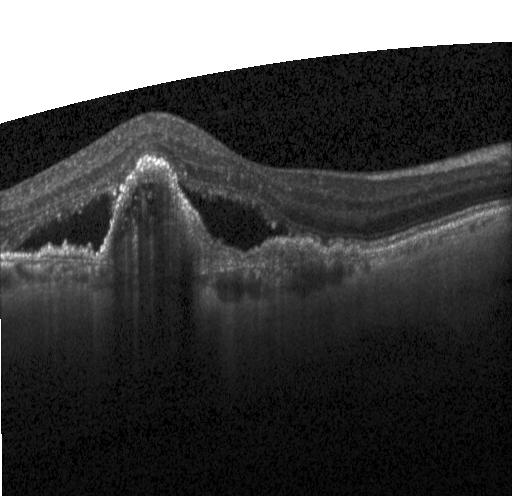

Spectral-domain optical coherence tomography; fovea-centered; OCT B-scan. OCT finding: a choroidal neovascular membrane.